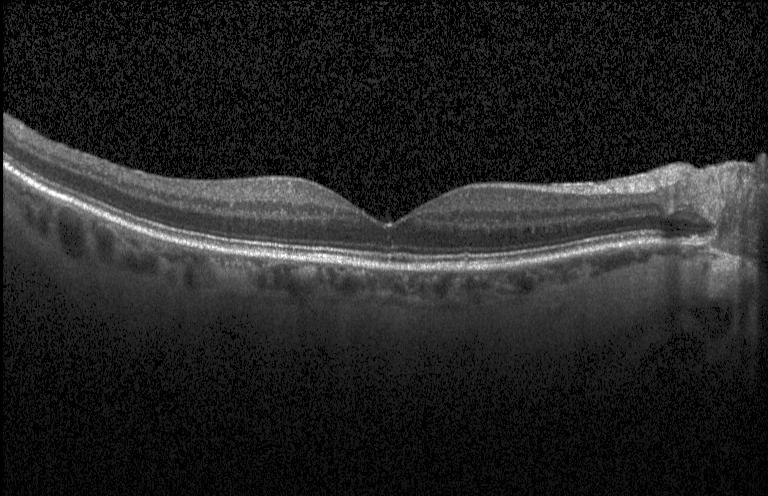 No choroidal neovascularization, diabetic macular edema, or drusen.